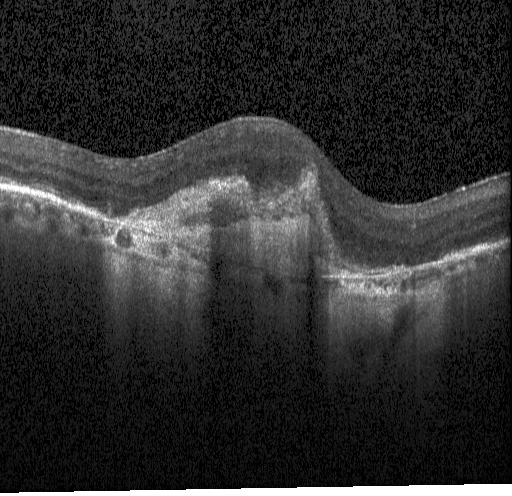 OCT B-scan, through the macula, spectral-domain OCT
Diagnosis: a choroidal neovascular membrane.